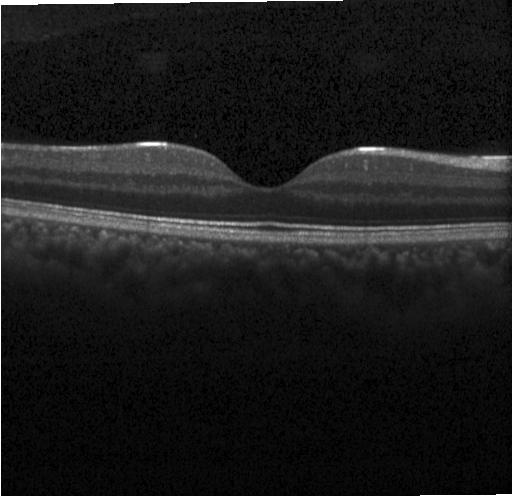
Optical coherence tomography scan; Heidelberg Spectralis OCT system; SD-OCT; through the macula — Diagnosis: no CNV, DME, or drusen.